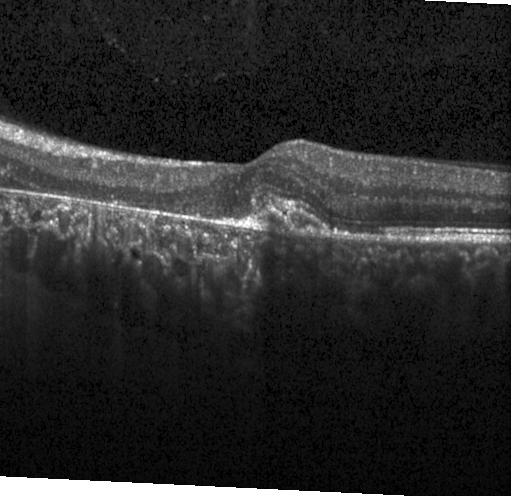 Retinal OCT cross-section showing a choroidal neovascular membrane.